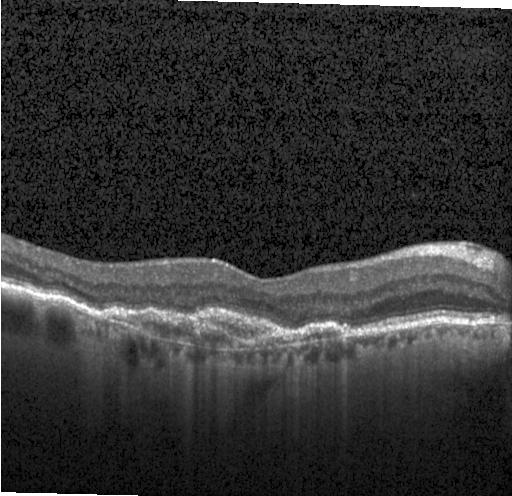
OCT B-scan — This B-scan demonstrates a choroidal neovascular membrane.